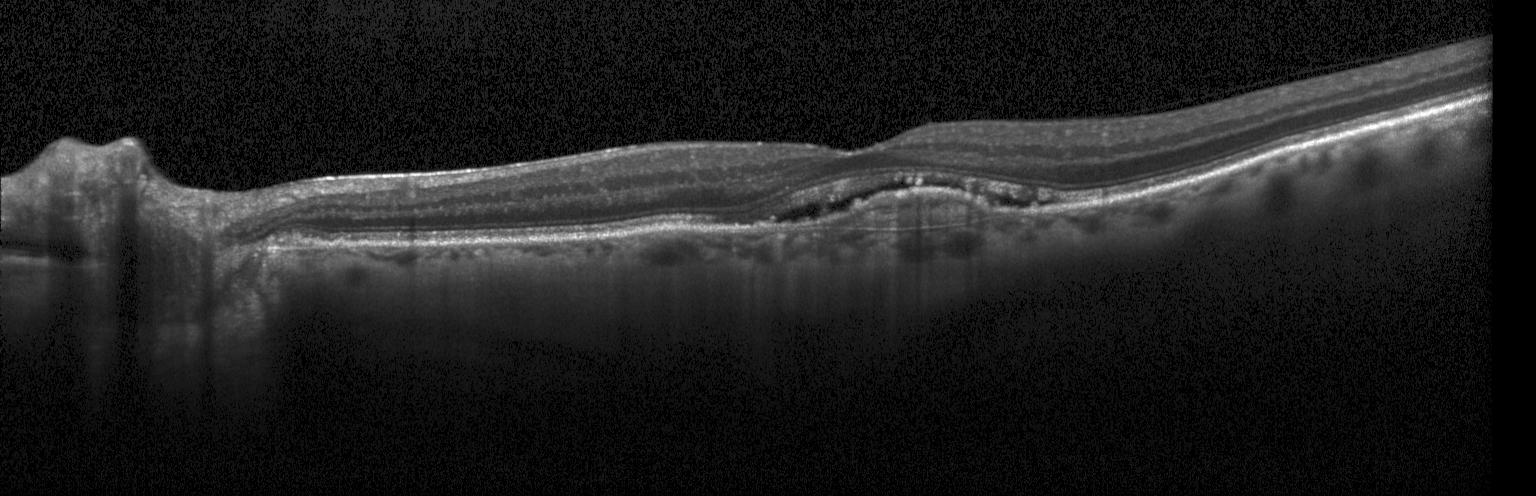
A choroidal neovascular membrane.